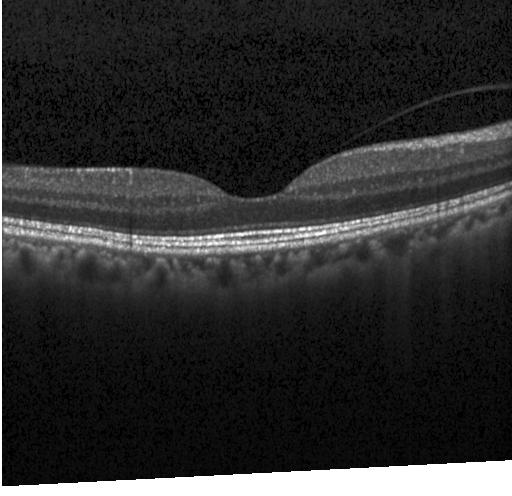 Centered on the fovea. OCT B-scan. SD-OCT. Macular OCT: no CNV, DME, or drusen.